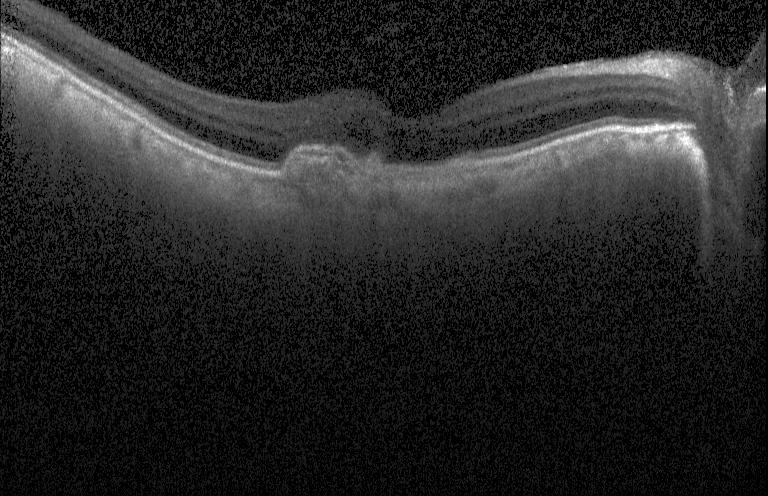

Finding: choroidal neovascularization.